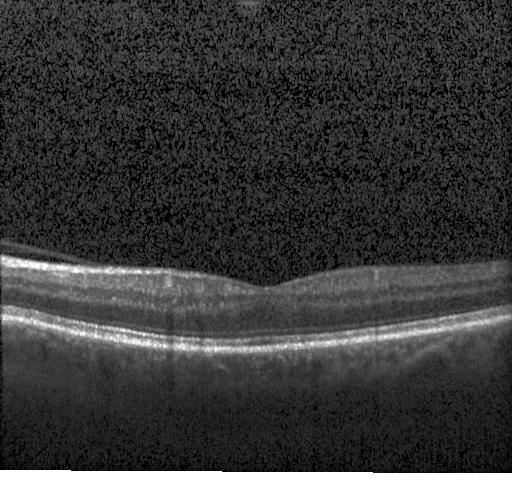
Macular OCT demonstrating no choroidal neovascularization, diabetic macular edema, or drusen.